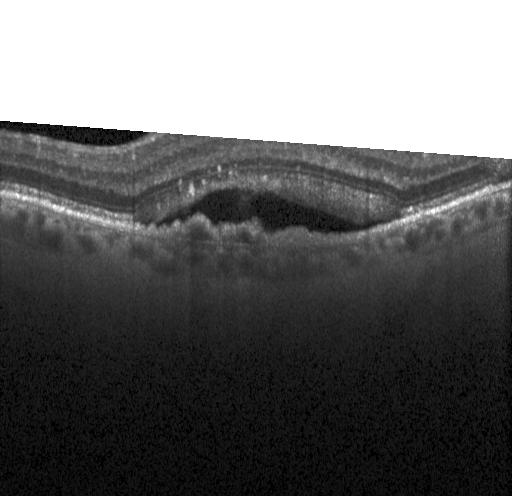 Heidelberg Spectralis; retinal OCT cross-section — This B-scan demonstrates a choroidal neovascular membrane.